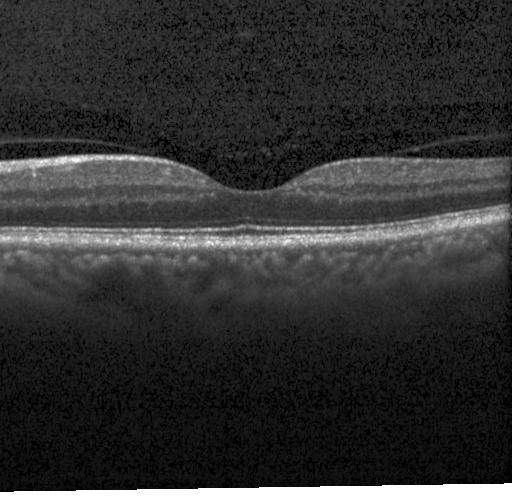

Assessment: neither CNV, DME, nor drusen.